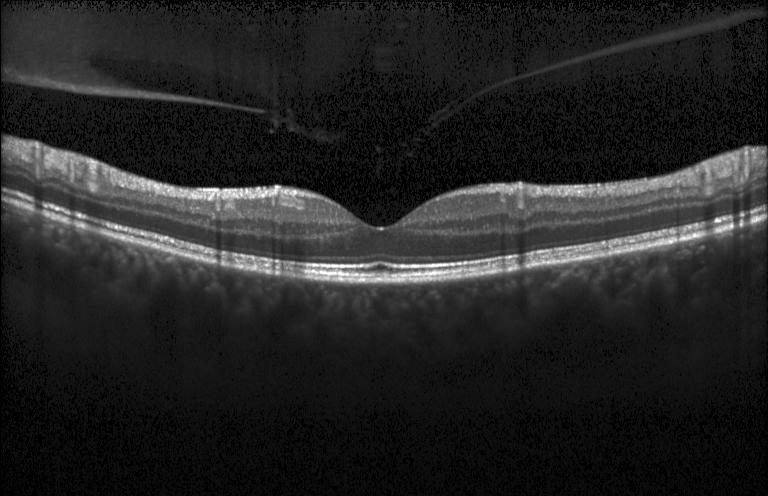

The scan shows neither choroidal neovascularization, diabetic macular edema, nor drusen.